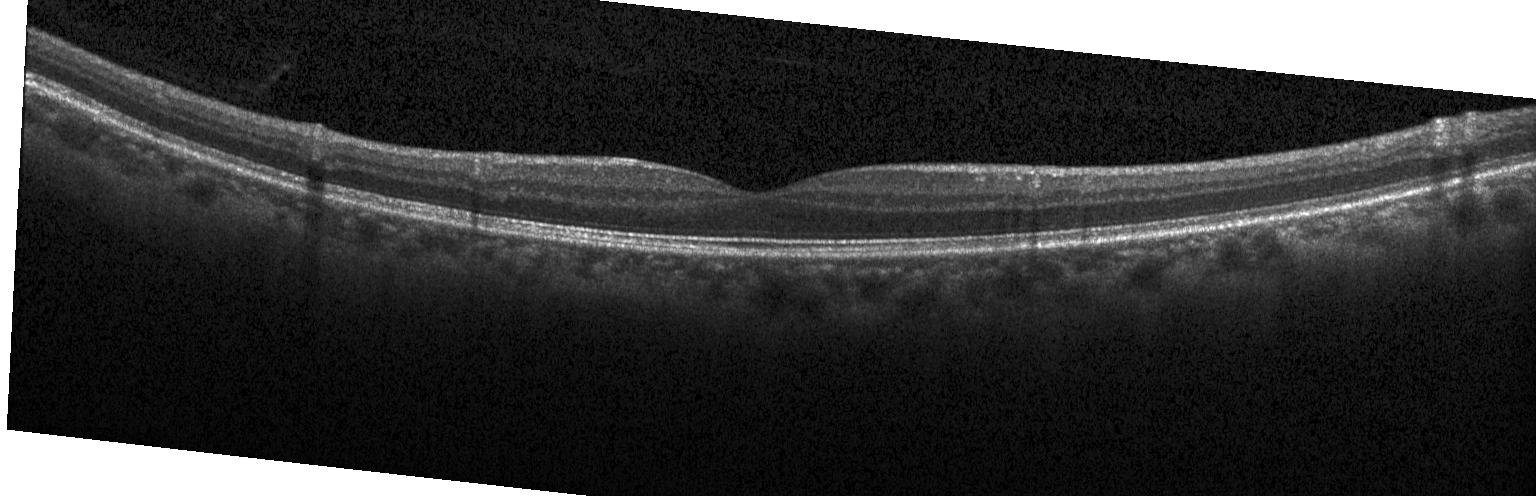

Spectral-domain optical coherence tomography; OCT B-scan
OCT finding: no evidence of CNV, DME, or drusen.